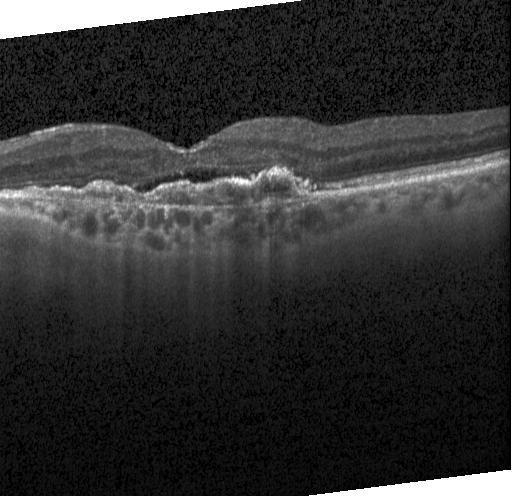
Fovea-centered, Heidelberg Spectralis OCT system, OCT B-scan. Diagnosis: a choroidal neovascular membrane.